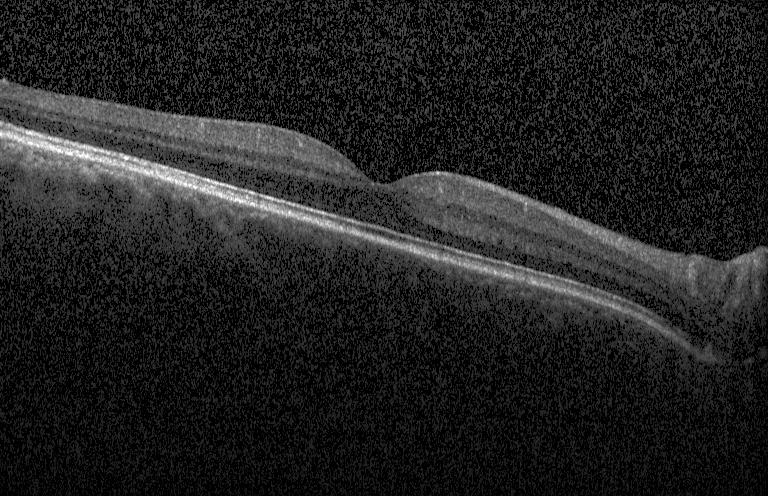

Impression: neither choroidal neovascularization, diabetic macular edema, nor drusen.